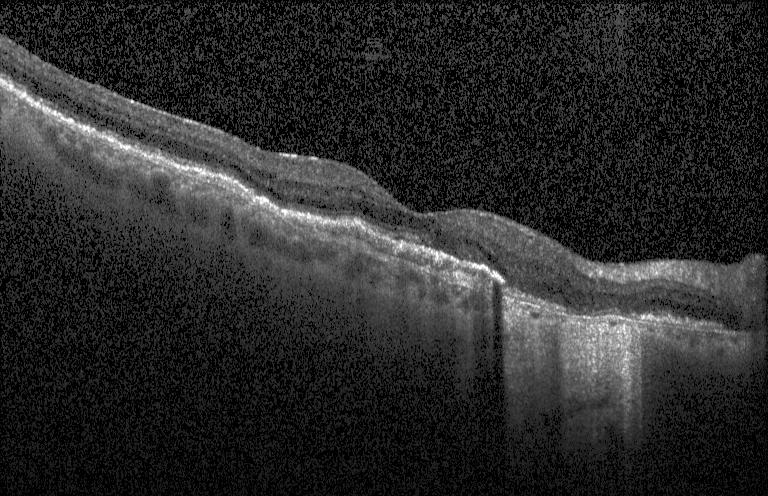
A choroidal neovascular membrane.